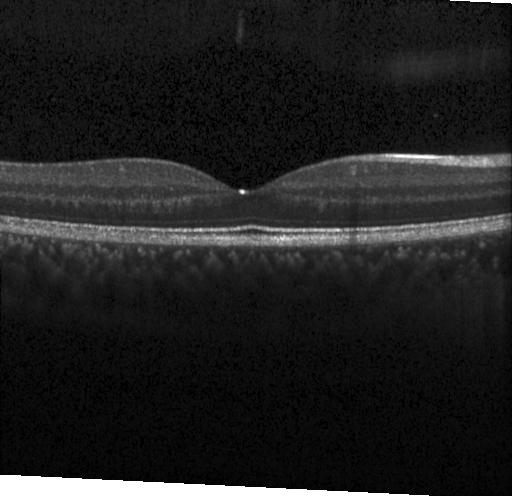
Dx: no choroidal neovascularization, no diabetic macular edema, and no drusen.